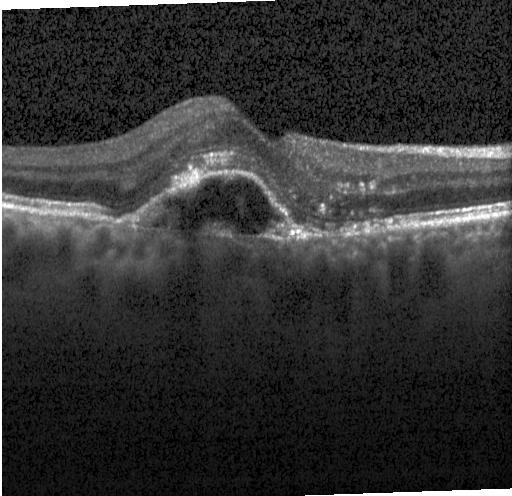
Macular OCT: choroidal neovascularization.